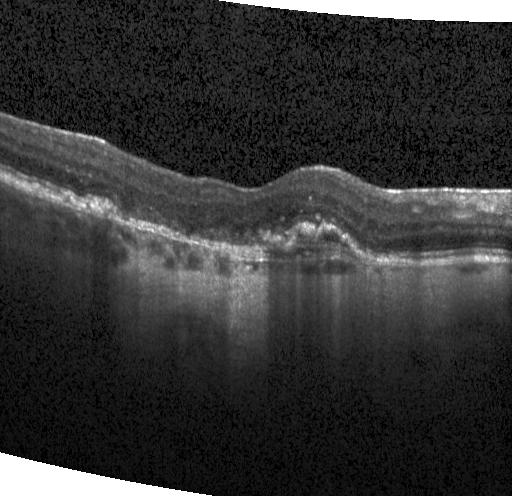

Spectral-domain OCT B-scan: a choroidal neovascular membrane.